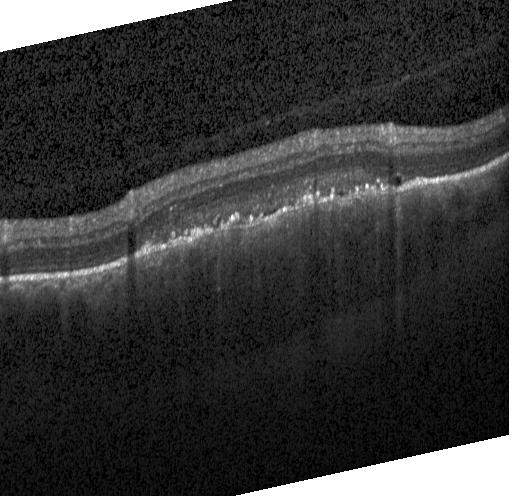 Finding: CNV.